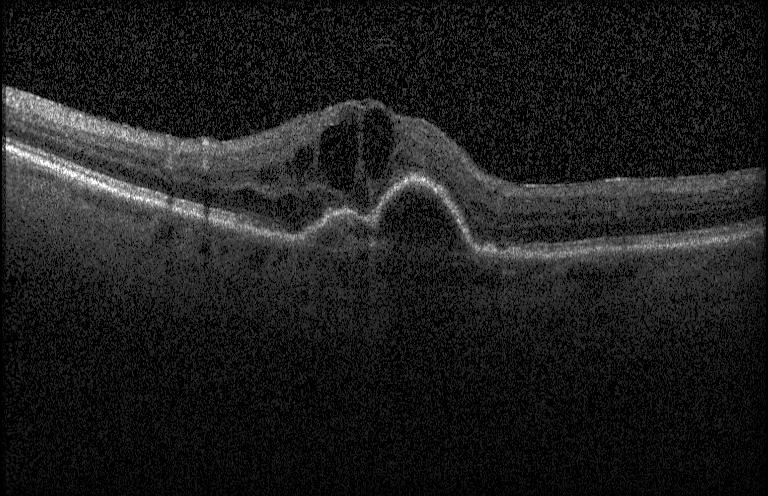
Spectral-domain OCT B-scan: a choroidal neovascular membrane.